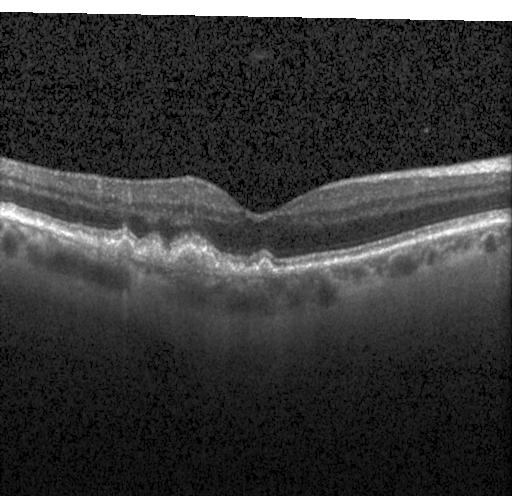

Acquired on a Heidelberg Spectralis; SD-OCT; OCT line scan; fovea-centered
Sub-RPE drusenoid deposits.